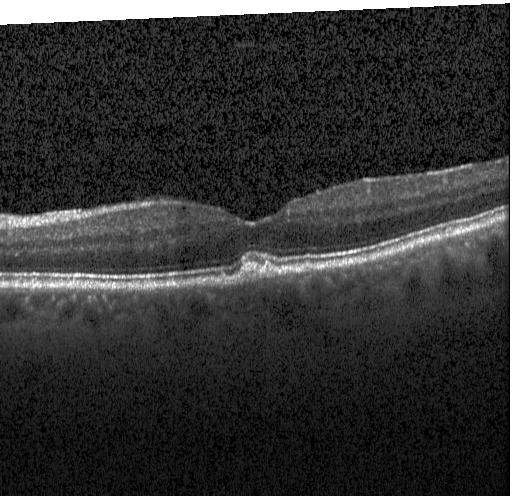
Macular OCT: sub-RPE drusenoid deposits.